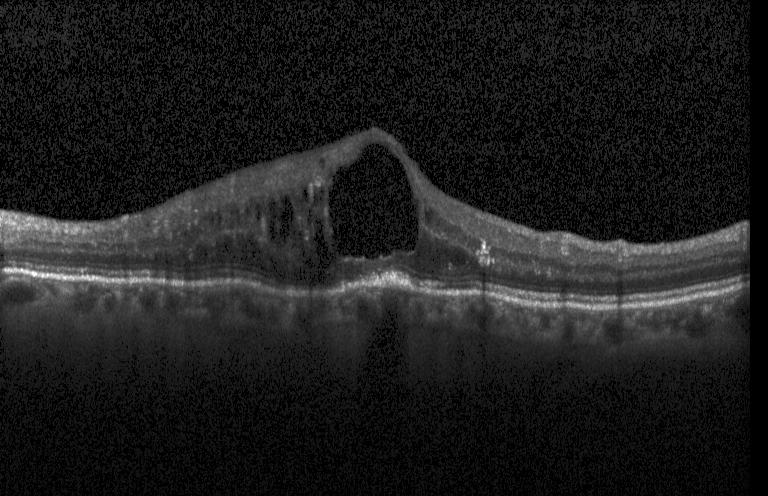

Centered on the fovea. Retinal OCT B-scan. Spectral-domain optical coherence tomography. Heidelberg Spectralis OCT system
DME.